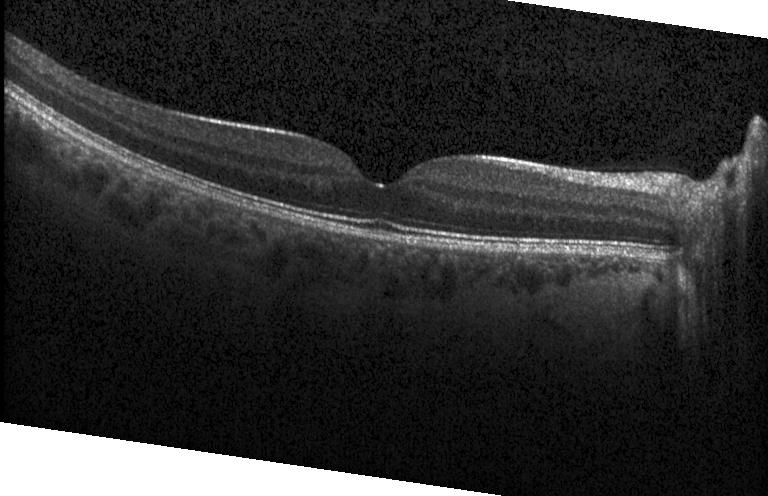

Retinal OCT cross-section
The scan shows neither CNV, DME, nor drusen.